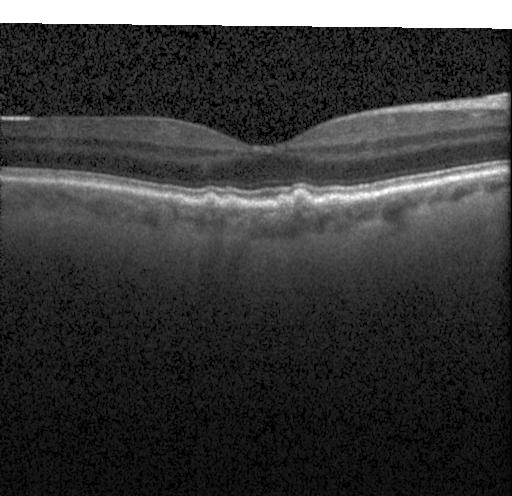 Macular OCT: sub-RPE drusenoid deposits.